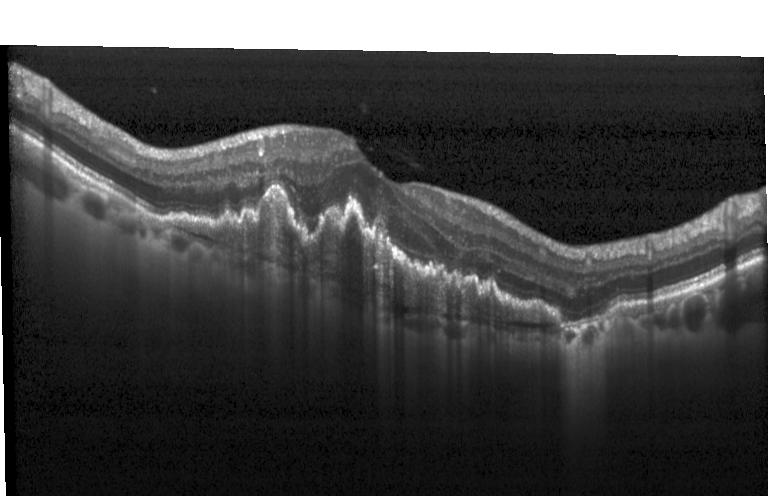 Optical coherence tomography scan
Impression: a choroidal neovascular membrane.